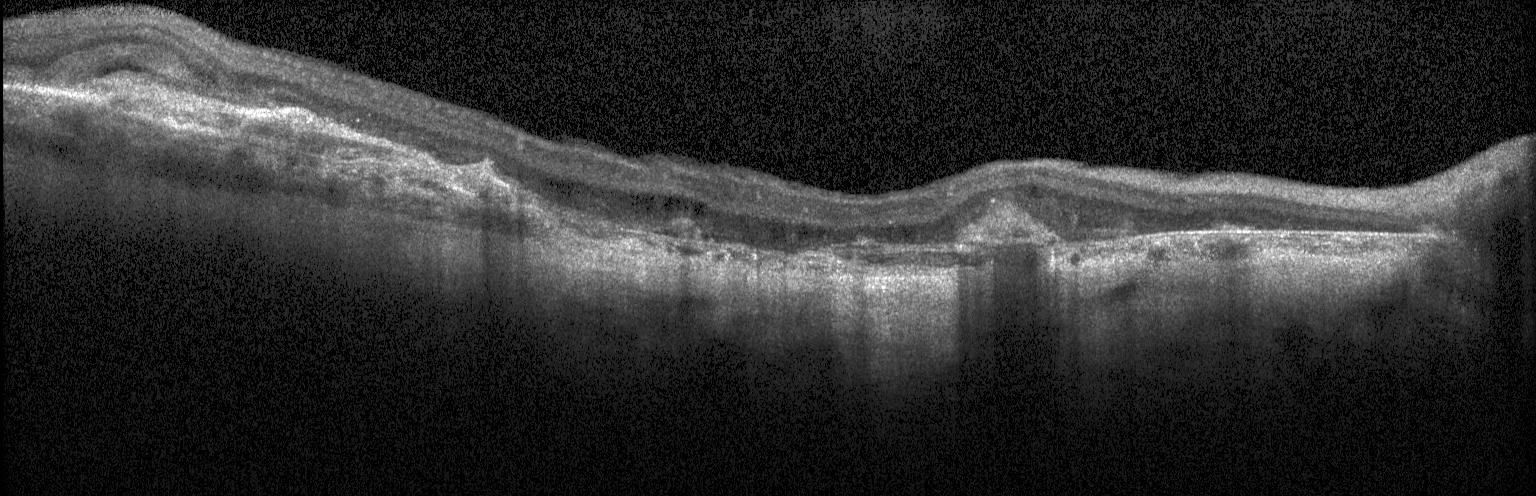
Acquired on a Heidelberg Spectralis · optical coherence tomography scan · spectral-domain OCT.
This B-scan demonstrates a choroidal neovascular membrane.